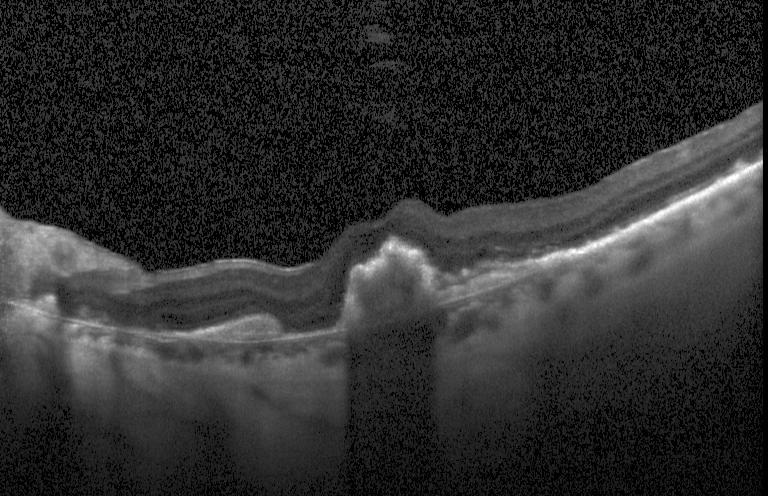

Retinal OCT cross-section — Diagnosis: a choroidal neovascular membrane.